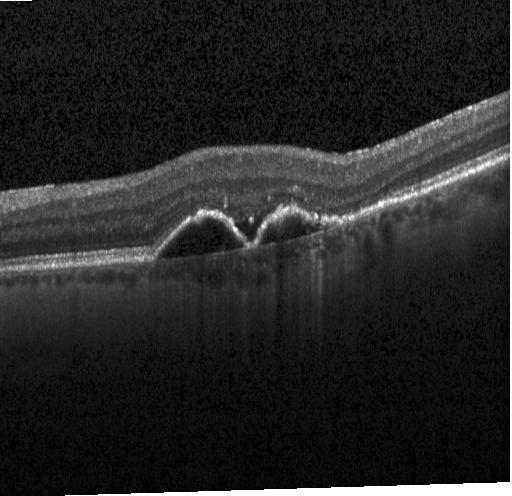
Spectral-domain optical coherence tomography. Fovea-centered. Instrument: Heidelberg Spectralis. Retinal OCT B-scan — Assessment: a choroidal neovascular membrane.